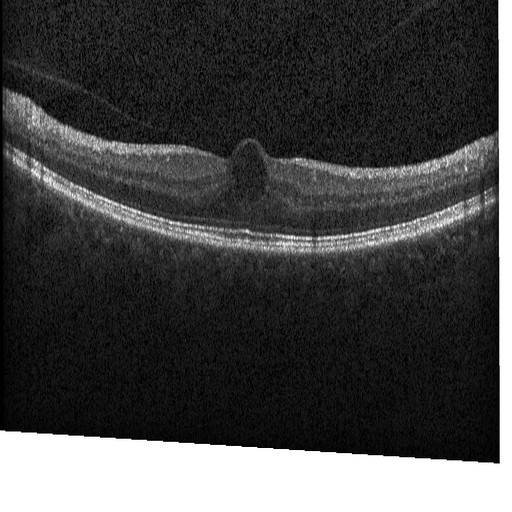
Macular OCT demonstrating DME.